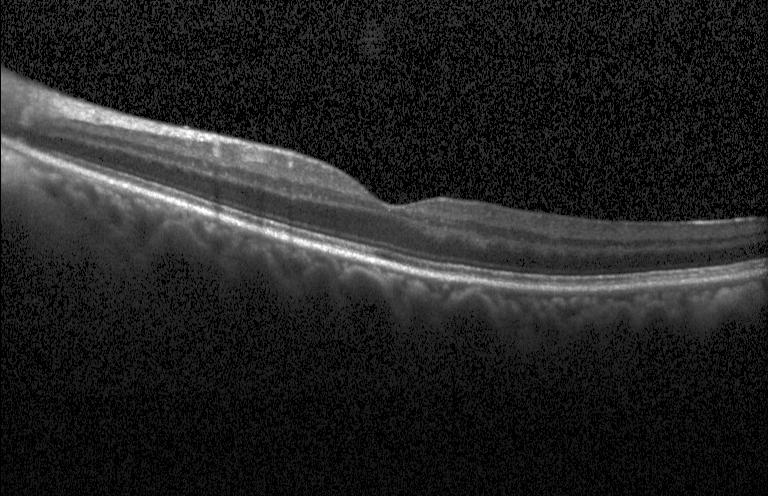 Retinal OCT cross-section.
Diagnosis: neither CNV, DME, nor drusen.